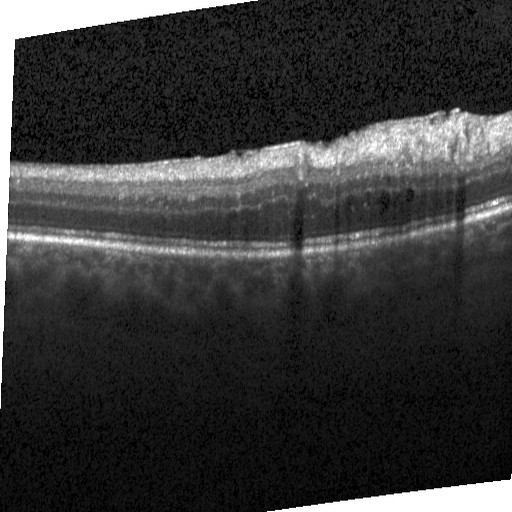
Retinal OCT B-scan — Finding: DME.